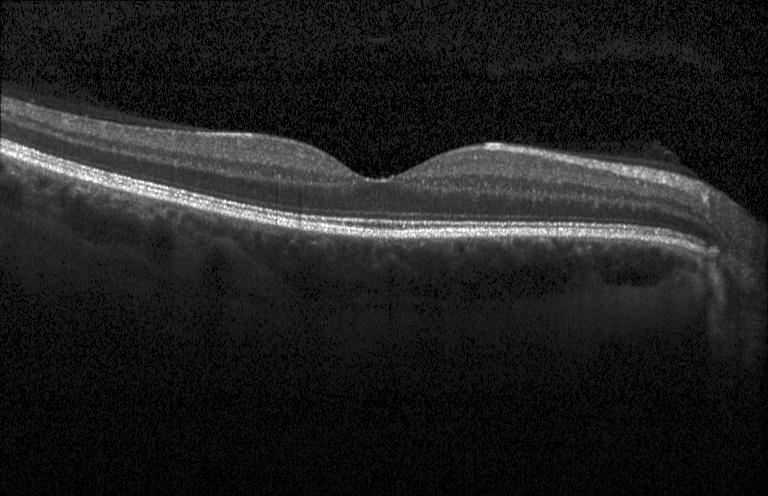

Finding: no CNV, DME, or drusen.